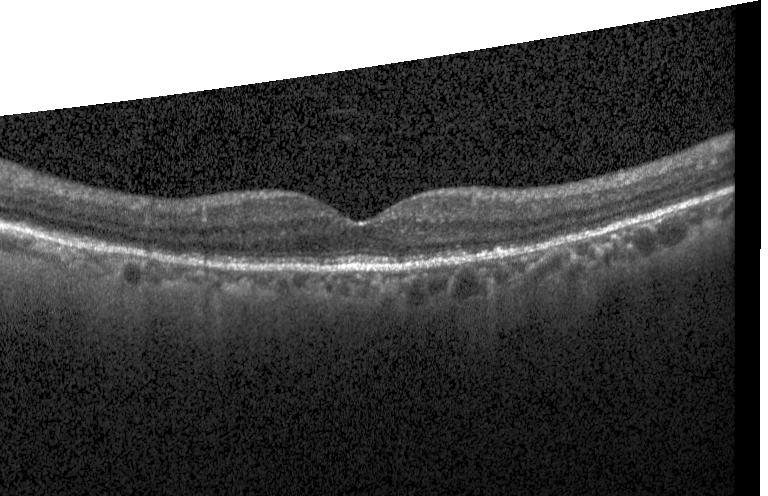

OCT scan showing no choroidal neovascularization, diabetic macular edema, or drusen.